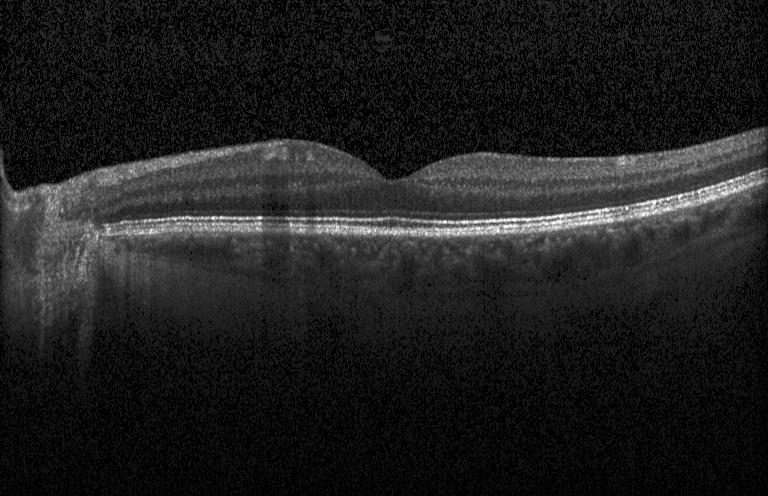 OCT B-scan.
Impression: no choroidal neovascularization, diabetic macular edema, or drusen.